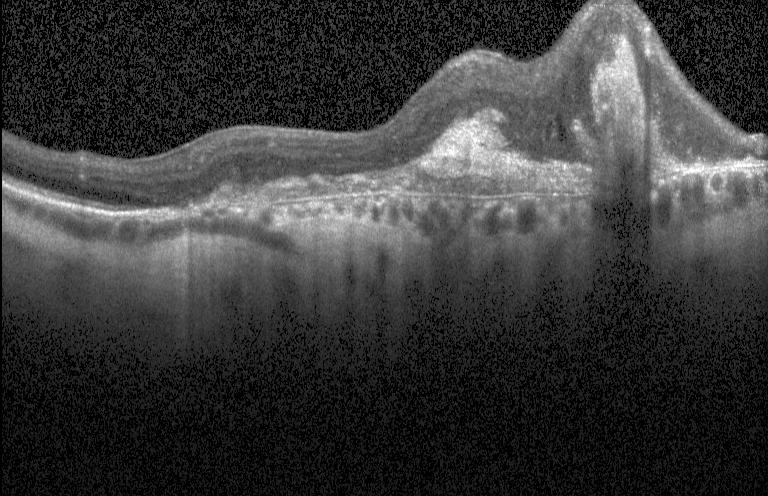

OCT scan showing a choroidal neovascular membrane.